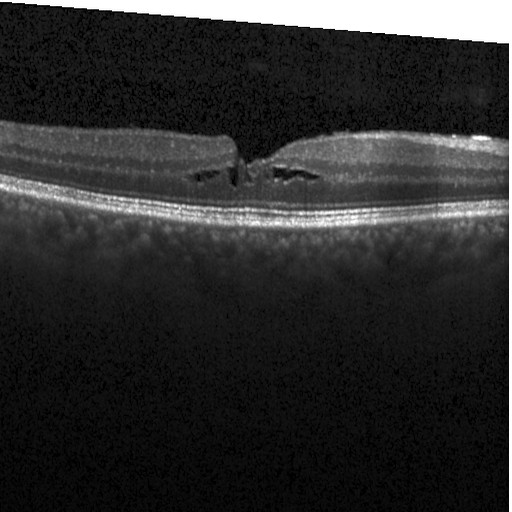
Optical coherence tomography B-scan. Heidelberg Spectralis. Spectral-domain OCT. Macular scan — Assessment: DME.